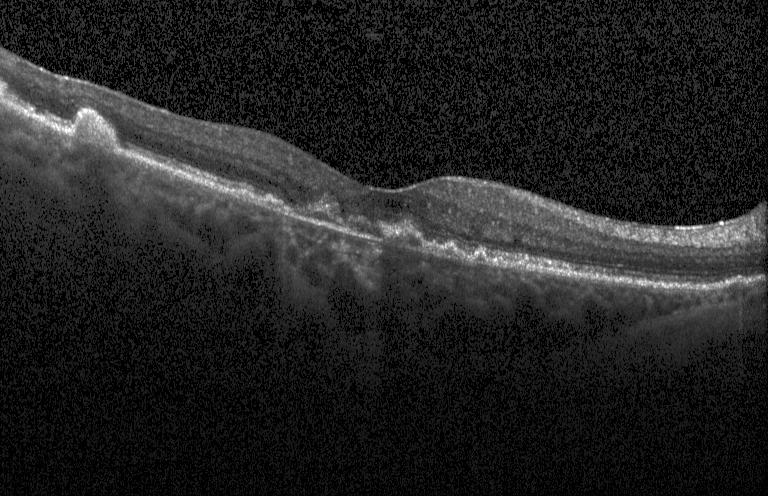 Retinal OCT B-scan — Assessment: a choroidal neovascular membrane.